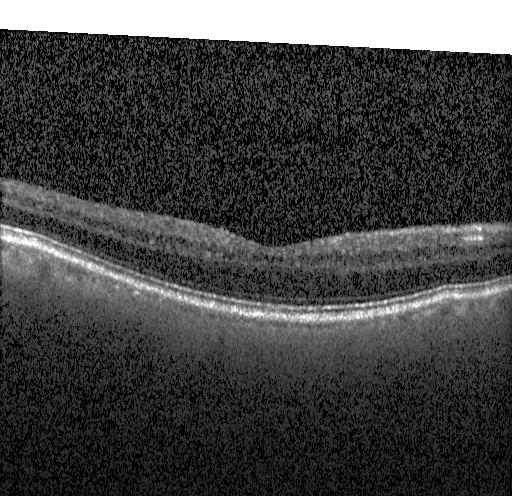

OCT B-scan; Heidelberg Spectralis OCT system; horizontal scan through the fovea; spectral-domain OCT.
This B-scan demonstrates neither CNV, DME, nor drusen.